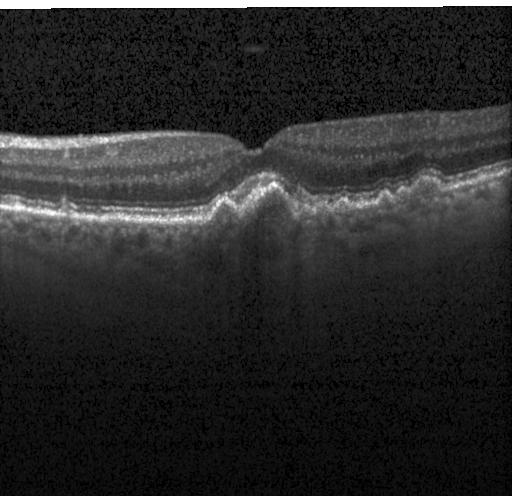

OCT B-scan. Heidelberg Spectralis
Impression: drusen.